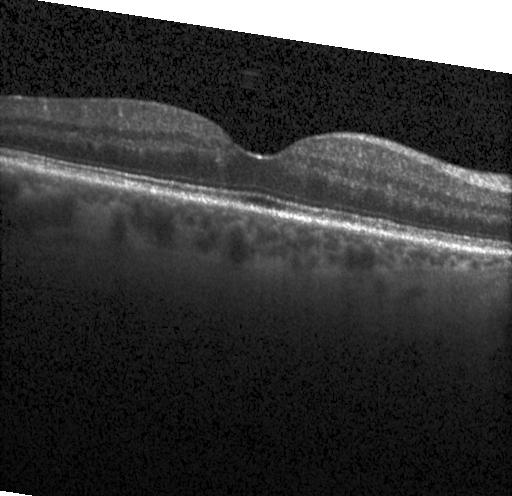 Neither CNV, DME, nor drusen.